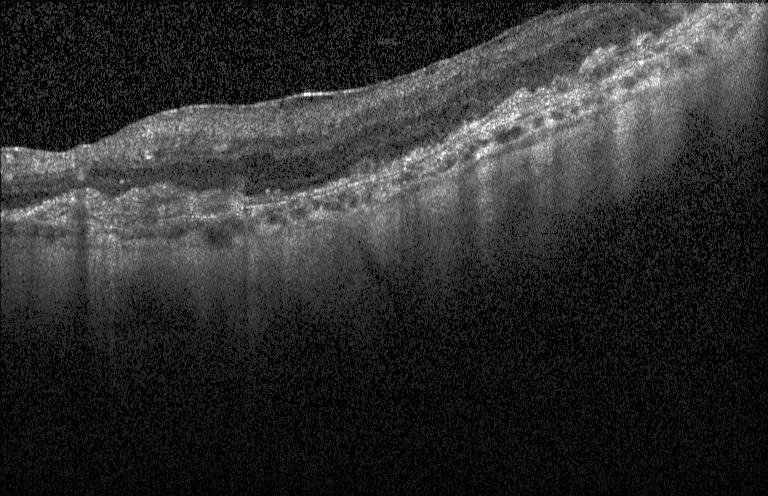
Macular OCT demonstrating CNV.